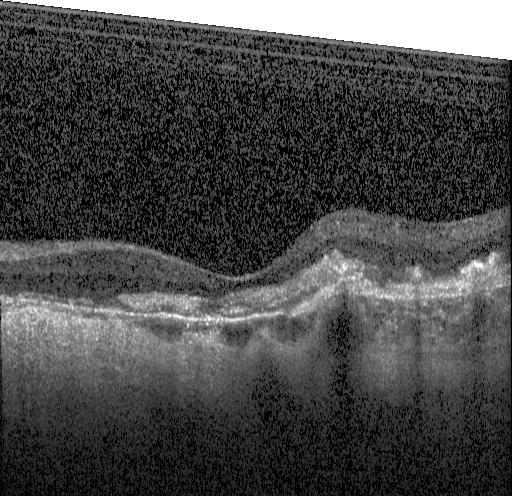 Acquired on a Heidelberg Spectralis. SD-OCT. OCT B-scan. Centered on the fovea — Finding: CNV.